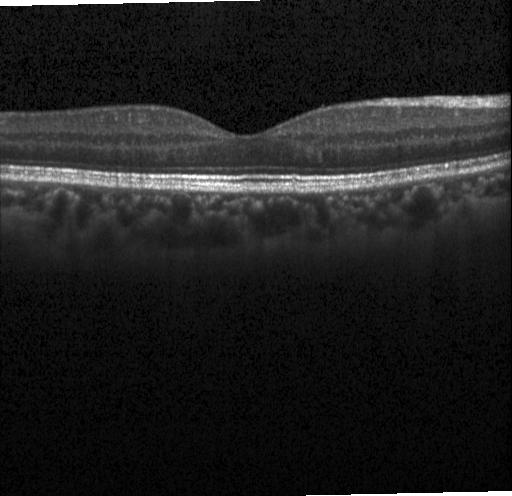

Spectral-domain optical coherence tomography, macular scan, OCT B-scan.
This B-scan demonstrates no evidence of CNV, DME, or drusen.